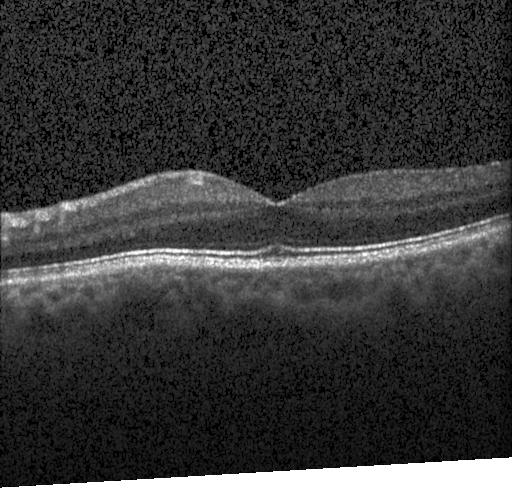
SD-OCT, through the macula, retinal OCT B-scan, Heidelberg Spectralis OCT system.
The scan shows neither choroidal neovascularization, diabetic macular edema, nor drusen.